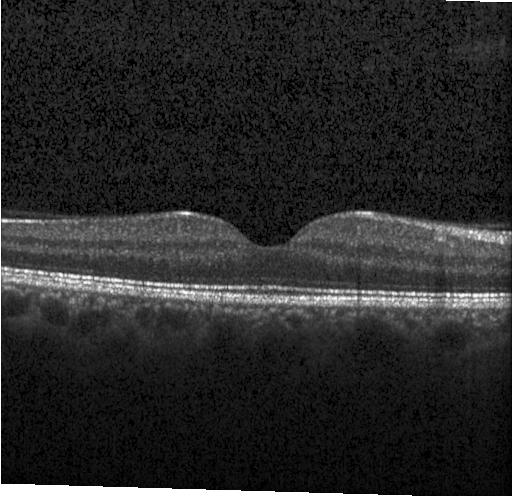
Fovea-centered · spectral-domain OCT · retinal OCT cross-section. Diagnosis: no choroidal neovascularization, diabetic macular edema, or drusen.